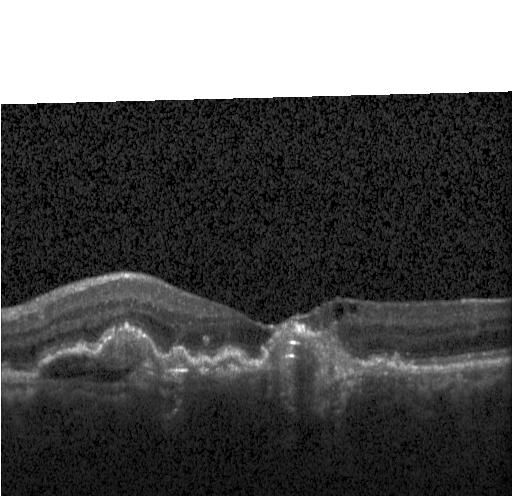
Optical coherence tomography scan
This B-scan demonstrates CNV.